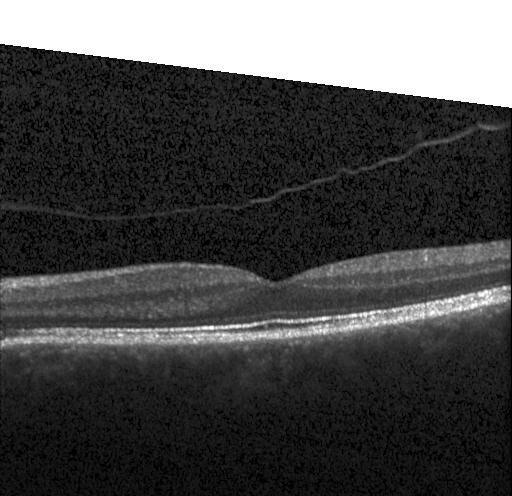 Impression: neither choroidal neovascularization, diabetic macular edema, nor drusen.